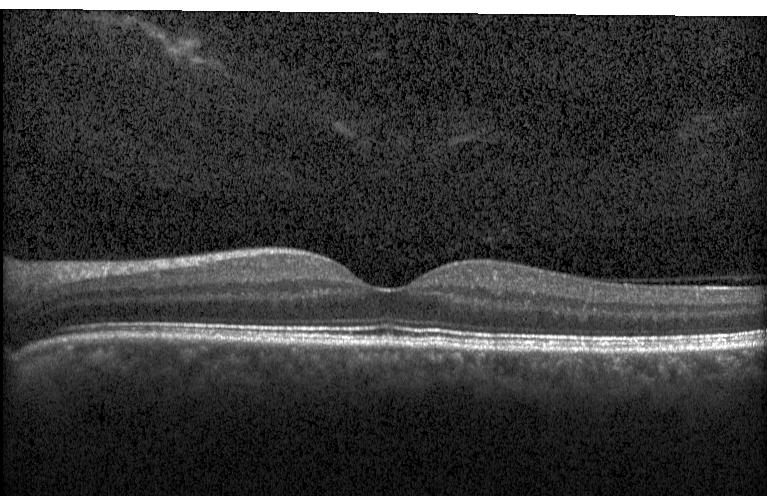
Horizontal scan through the fovea. OCT B-scan. Heidelberg Spectralis. Spectral-domain optical coherence tomography — Impression: neither choroidal neovascularization, diabetic macular edema, nor drusen.